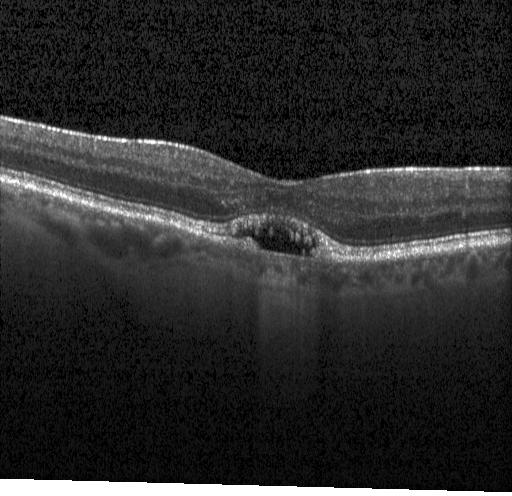

SD-OCT. Heidelberg Spectralis OCT system. Retinal OCT B-scan. Macular scan. Macular OCT: CNV.